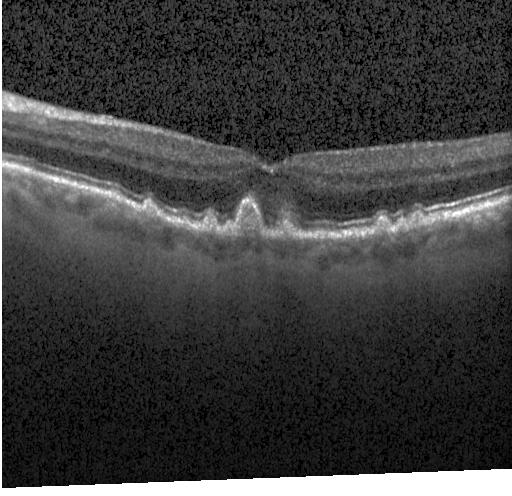 Retinal OCT B-scan, Heidelberg Spectralis OCT system, SD-OCT, through the macula.
The scan shows multiple drusen.